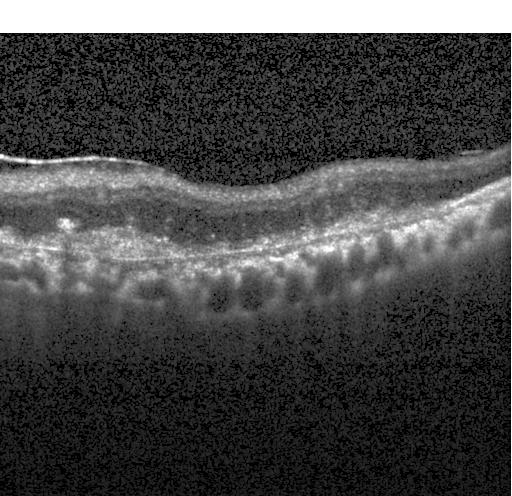
Spectral-domain OCT B-scan: a choroidal neovascular membrane.